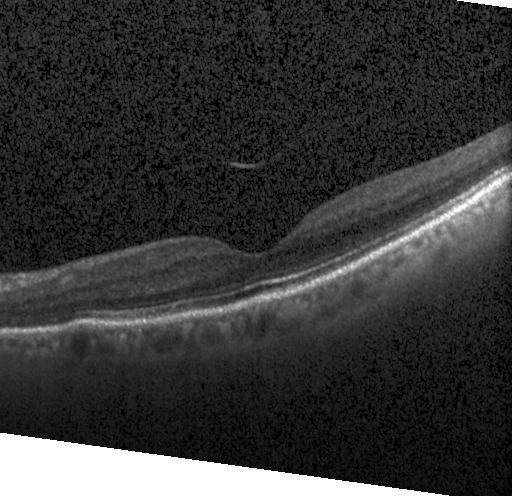

Through the macula · retinal OCT B-scan. Diagnosis: no choroidal neovascularization, diabetic macular edema, or drusen.